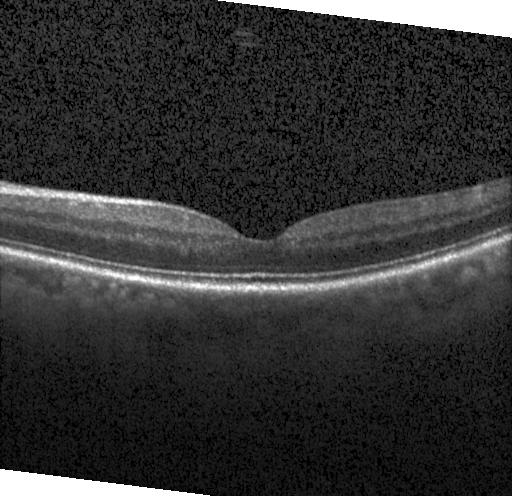
SD-OCT. Retinal OCT cross-section. Acquired on a Heidelberg Spectralis. This B-scan demonstrates no choroidal neovascularization, no diabetic macular edema, and no drusen.